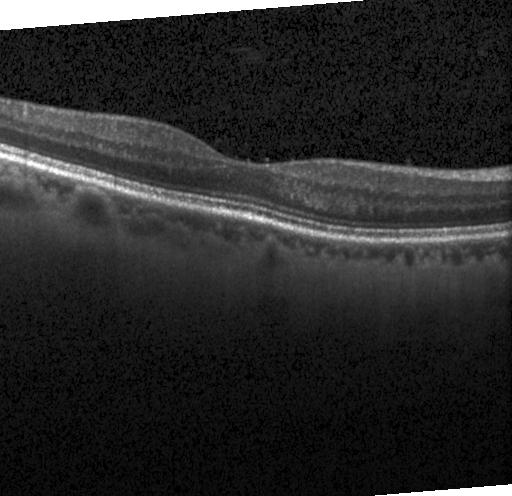
Instrument: Heidelberg Spectralis, macular scan, retinal OCT B-scan, spectral-domain OCT
Diagnosis: neither choroidal neovascularization, diabetic macular edema, nor drusen.